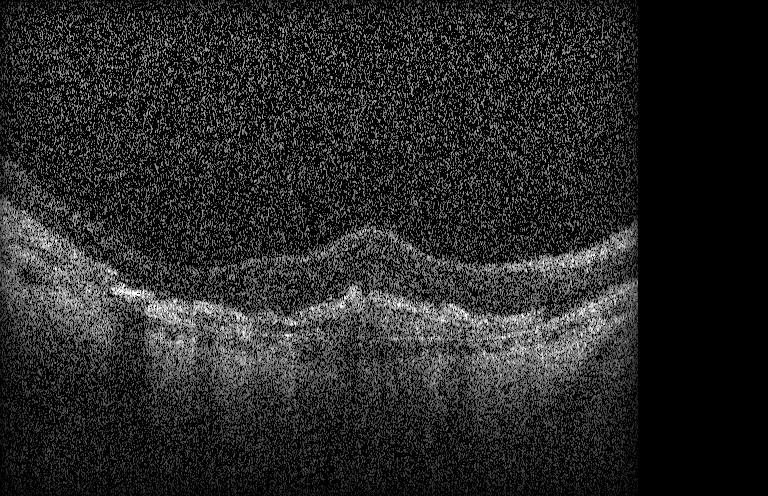

OCT B-scan
Impression: a choroidal neovascular membrane.